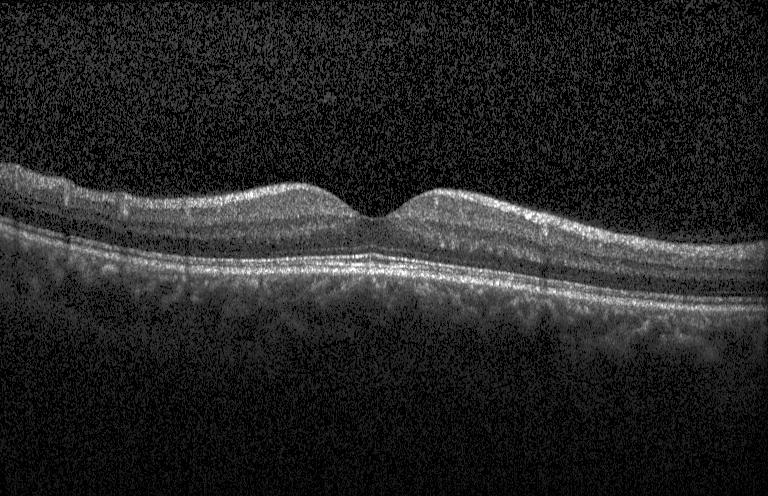
OCT B-scan.
This B-scan demonstrates neither choroidal neovascularization, diabetic macular edema, nor drusen.